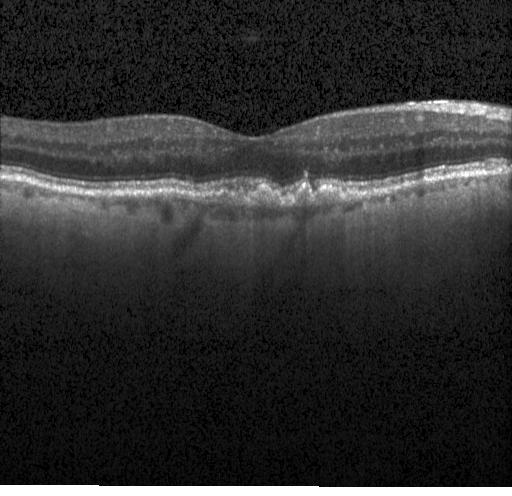
Spectral-domain OCT B-scan: sub-RPE drusenoid deposits.